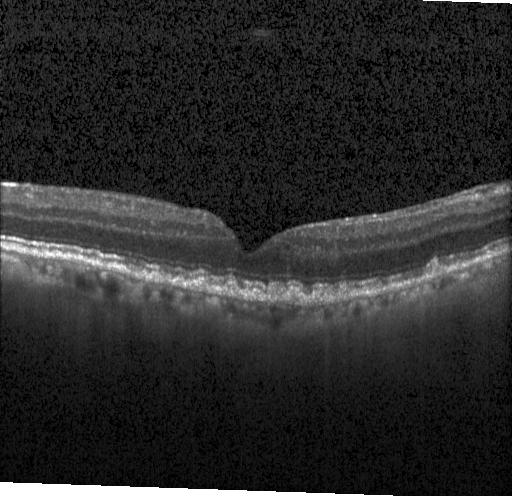

Optical coherence tomography B-scan.
Assessment: sub-RPE drusenoid deposits.